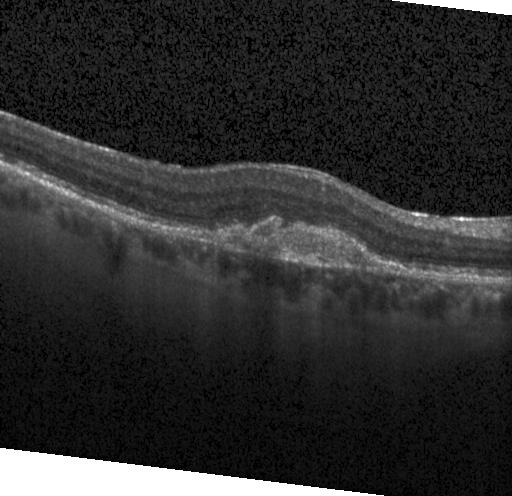

Retinal OCT cross-section. A choroidal neovascular membrane.